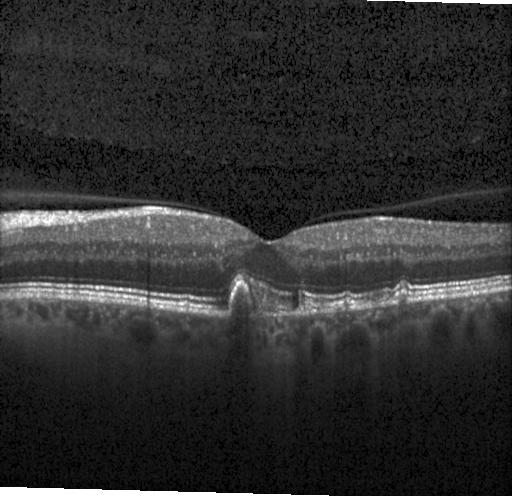 SD-OCT, Heidelberg Spectralis OCT system, retinal OCT cross-section. Impression: multiple drusen.